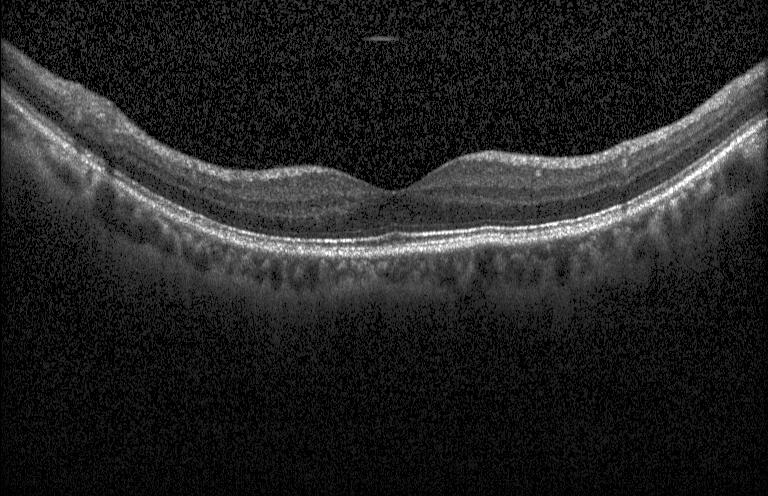 Finding: no evidence of choroidal neovascularization, diabetic macular edema, or drusen.